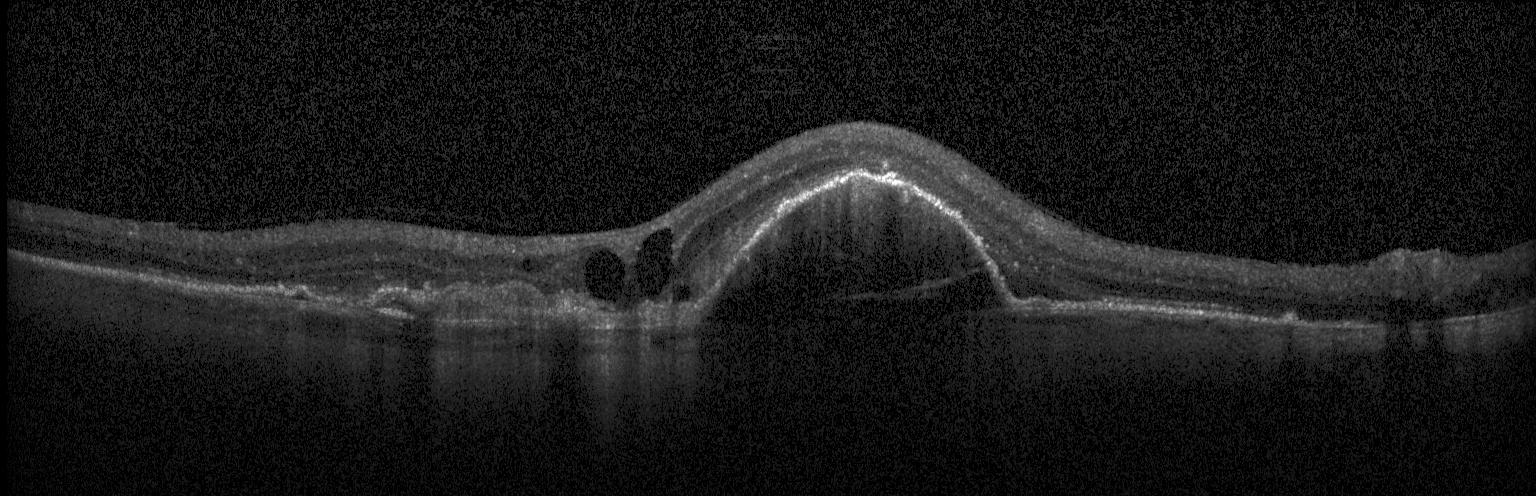

SD-OCT. OCT line scan. Fovea-centered. Heidelberg Spectralis OCT system.
Finding: choroidal neovascularization (CNV).